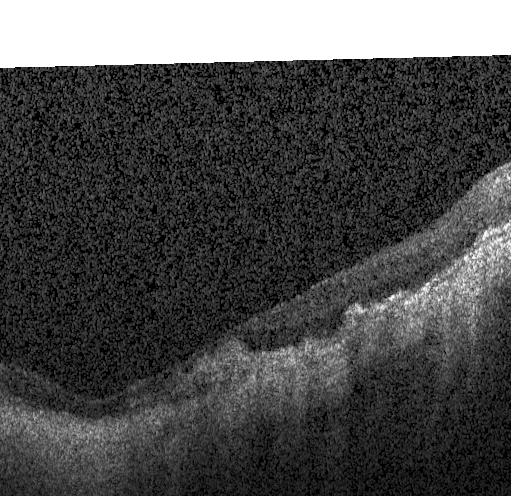
Macular OCT demonstrating a choroidal neovascular membrane.